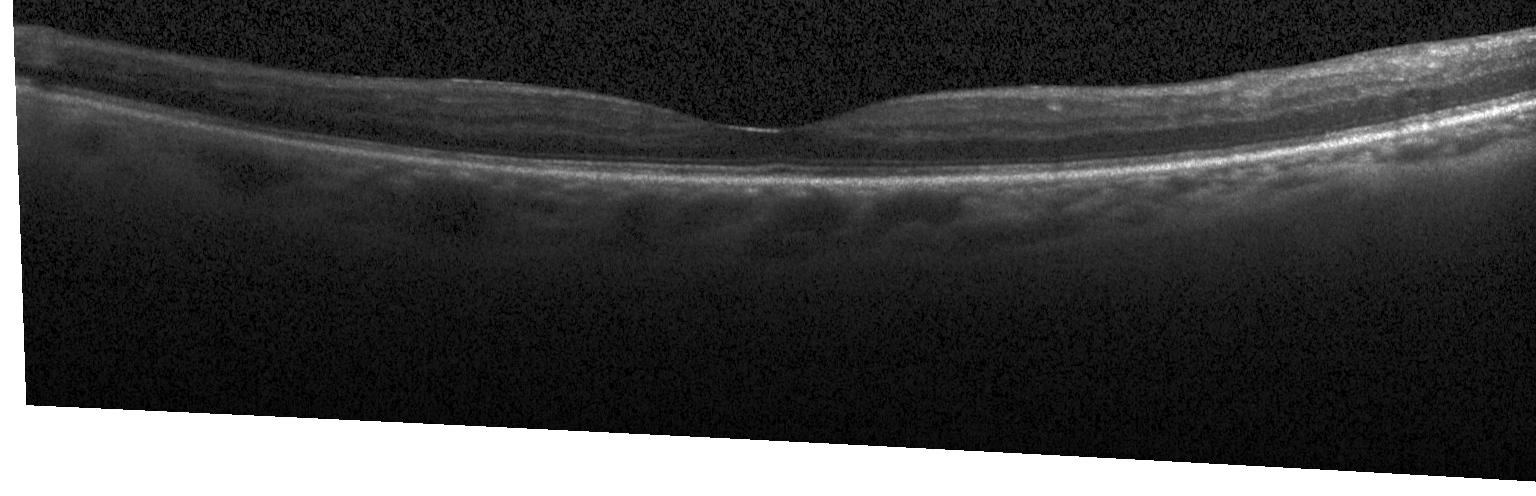
OCT finding: neither choroidal neovascularization, diabetic macular edema, nor drusen.